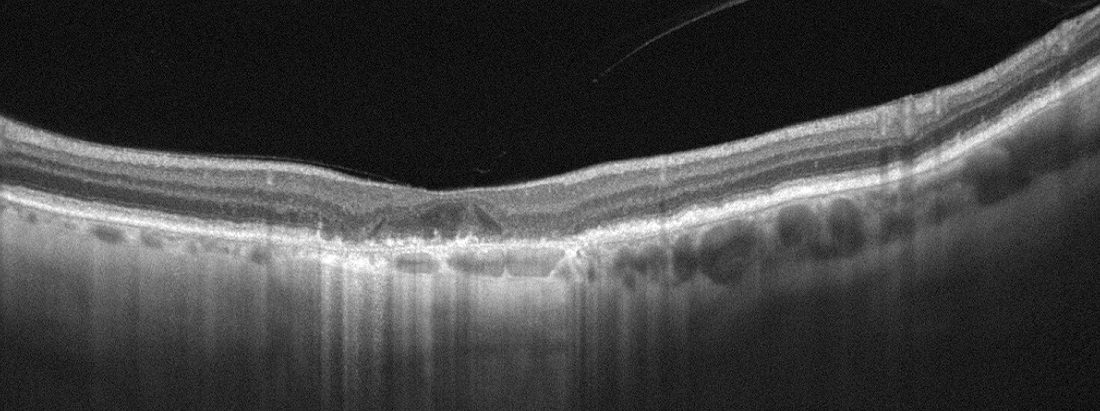

Retinal OCT cross-section — Impression: AMD.